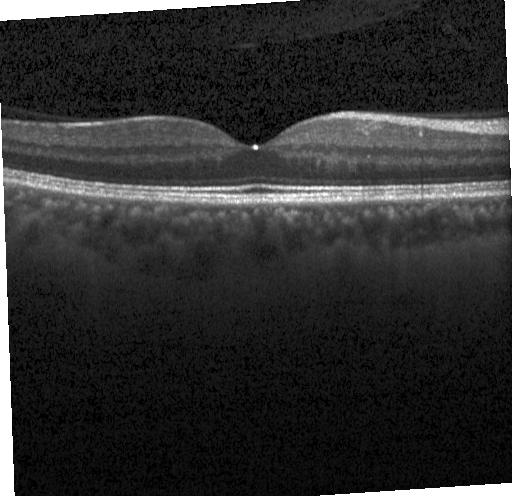
Fovea-centered · retinal OCT B-scan · Heidelberg Spectralis OCT system · SD-OCT
Diagnosis: no evidence of choroidal neovascularization, diabetic macular edema, or drusen.